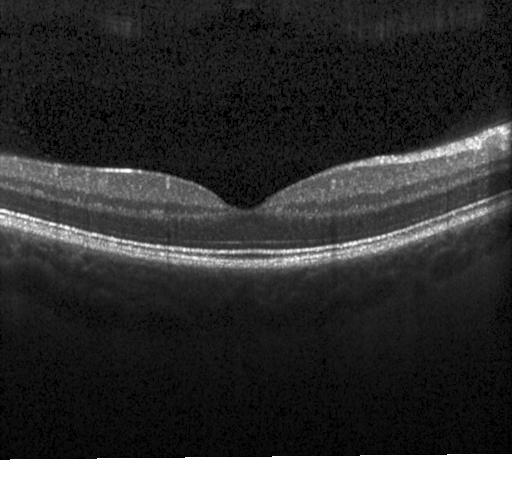 Heidelberg Spectralis OCT system, horizontal scan through the fovea, OCT line scan, SD-OCT.
Impression: neither CNV, DME, nor drusen.